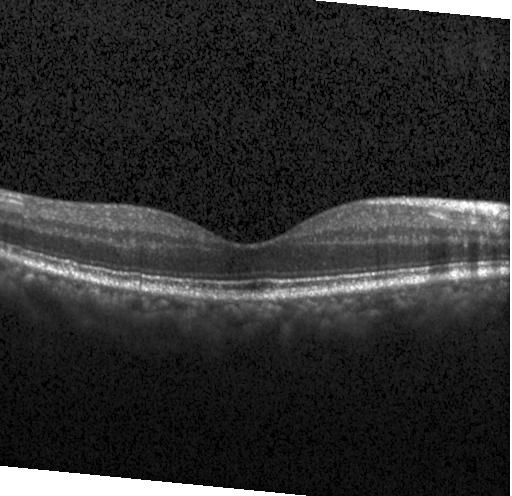 Centered on the fovea. Spectral-domain optical coherence tomography. OCT line scan. Impression: no choroidal neovascularization, no diabetic macular edema, and no drusen.